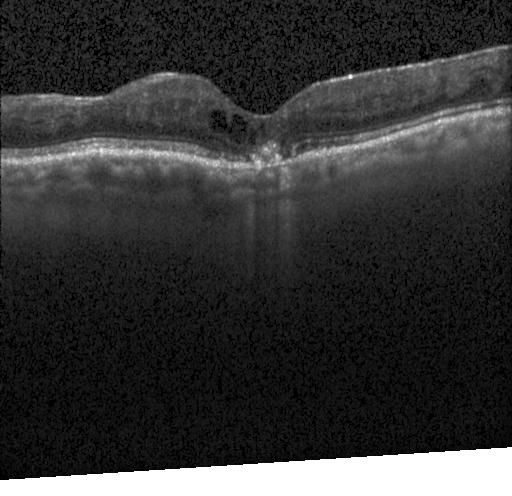 The scan shows a choroidal neovascular membrane.